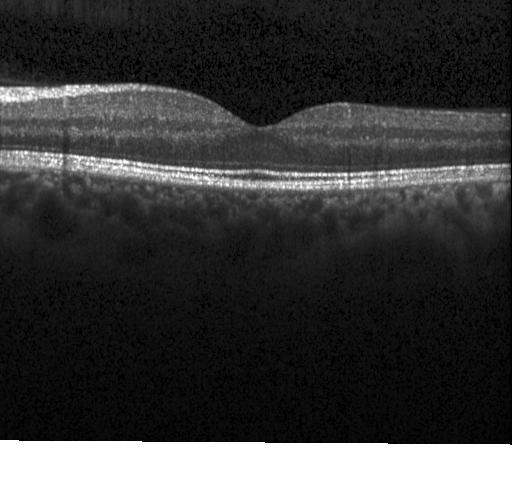 OCT line scan — This B-scan demonstrates no evidence of CNV, DME, or drusen.